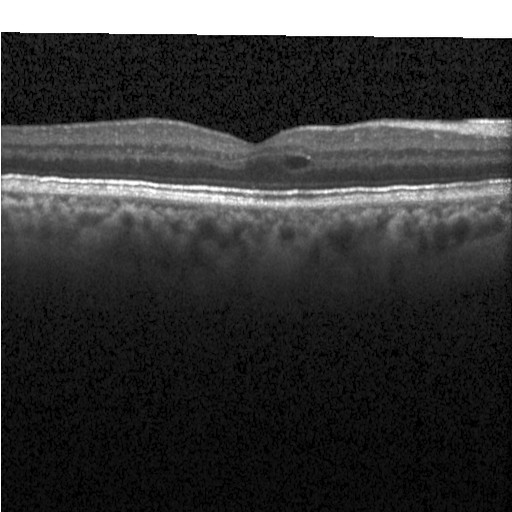 Assessment: diabetic macular edema (DME).